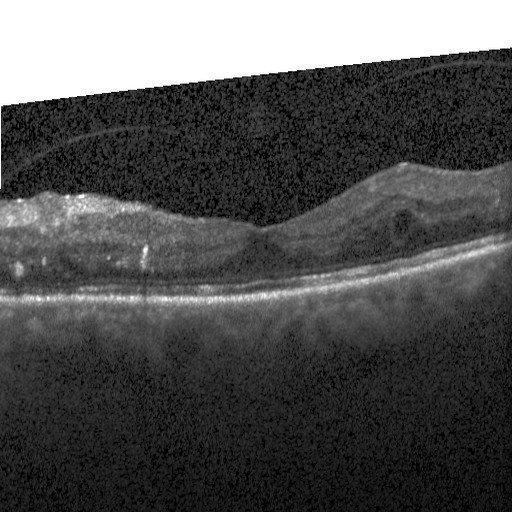

Retinal OCT B-scan
Finding: diabetic macular edema (DME).